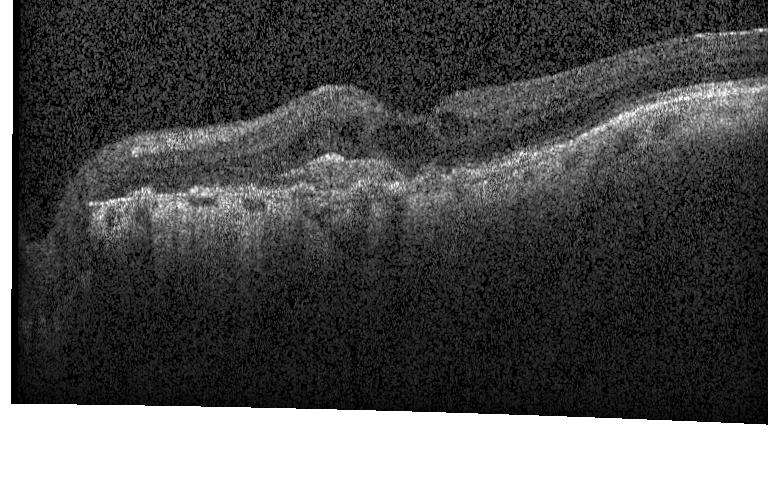 Heidelberg Spectralis OCT system. OCT line scan. SD-OCT. Fovea-centered.
Impression: a choroidal neovascular membrane.